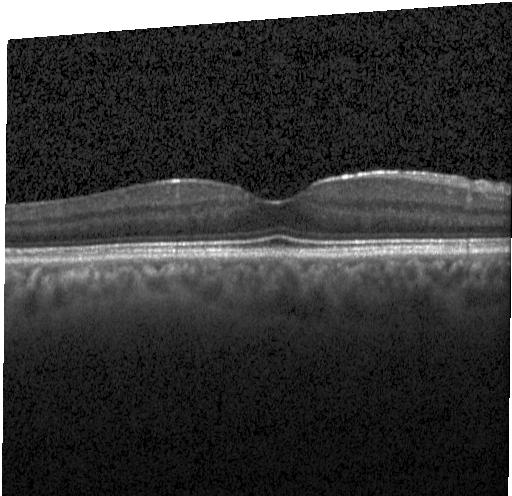
Diagnosis: no choroidal neovascularization, diabetic macular edema, or drusen.